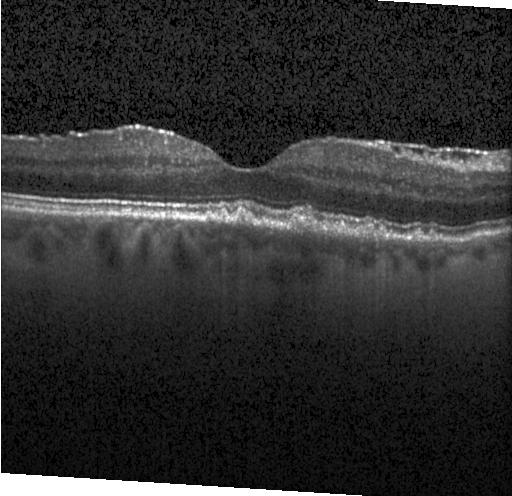
Macular scan; optical coherence tomography B-scan; spectral-domain OCT; Heidelberg Spectralis OCT system
Impression: drusen.